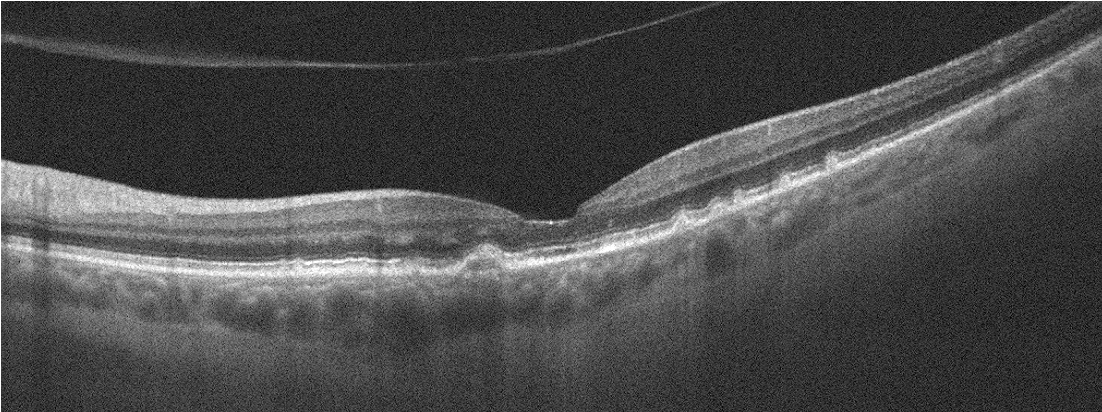

The scan shows age-related macular degeneration.